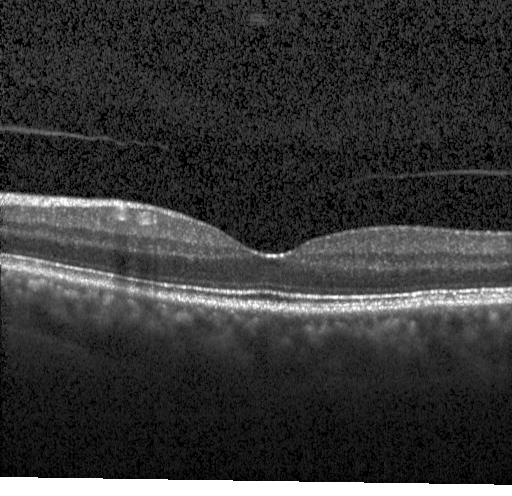

Optical coherence tomography scan — No CNV, no DME, and no drusen.